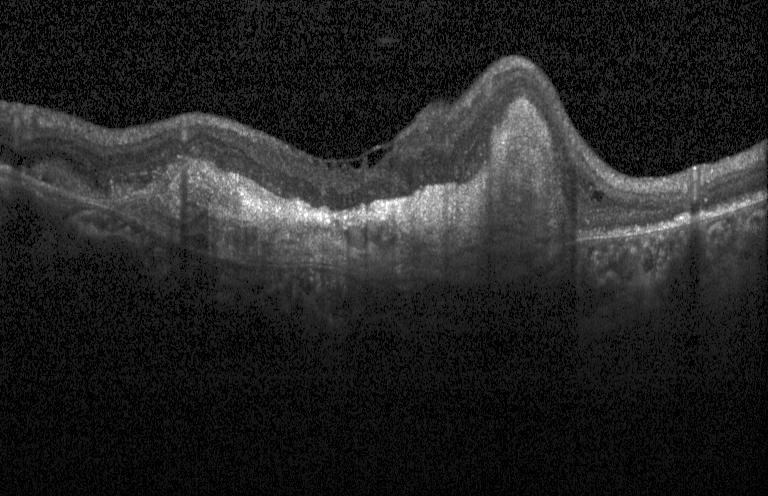
Choroidal neovascularization (CNV).